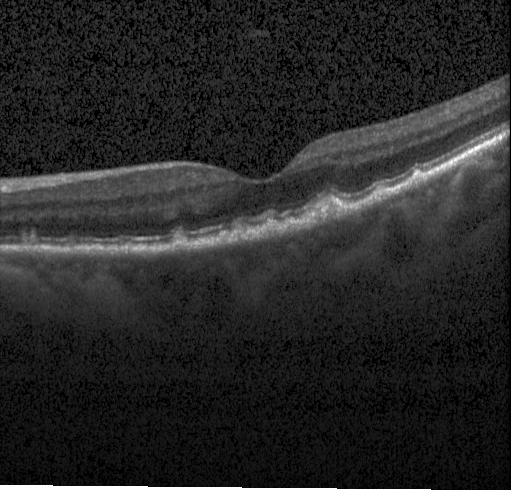
Optical coherence tomography B-scan, fovea-centered, Heidelberg Spectralis OCT system, spectral-domain optical coherence tomography.
Diagnosis: sub-RPE drusenoid deposits.